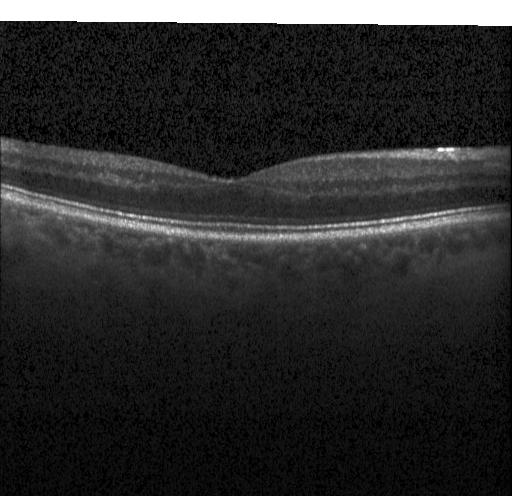 Impression: no evidence of CNV, DME, or drusen.